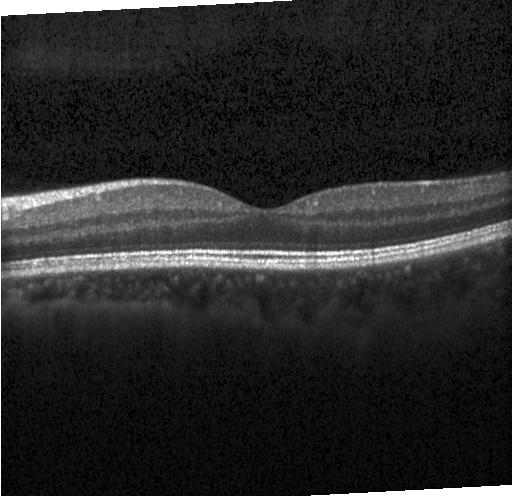

OCT B-scan
No CNV, DME, or drusen.